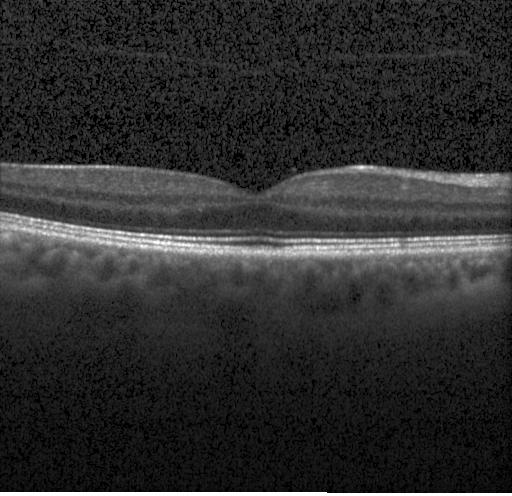 SD-OCT, instrument: Heidelberg Spectralis, retinal OCT B-scan, centered on the fovea
Impression: no choroidal neovascularization, no diabetic macular edema, and no drusen.